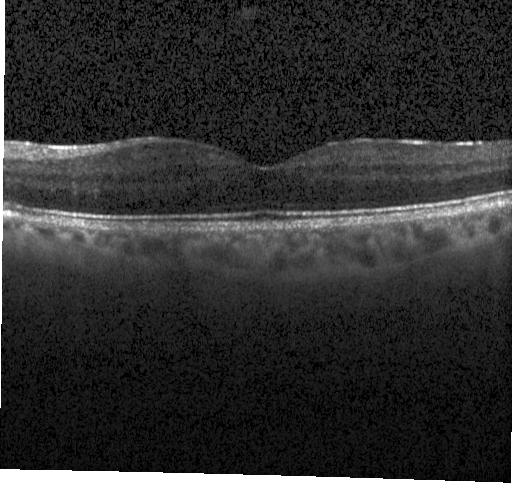
Optical coherence tomography scan — OCT finding: no choroidal neovascularization, no diabetic macular edema, and no drusen.